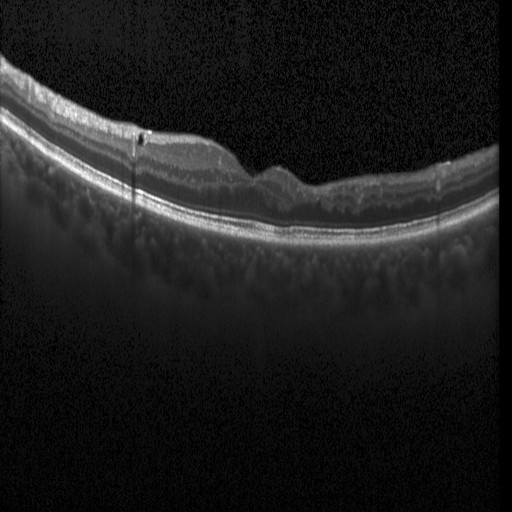

SD-OCT, Heidelberg Spectralis OCT system, optical coherence tomography scan — Finding: diabetic macular edema.